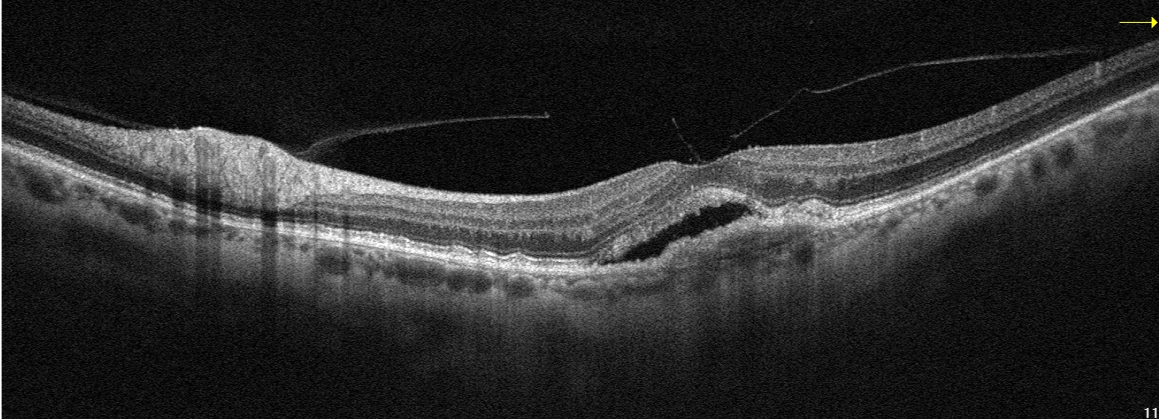 Dx: AMD.